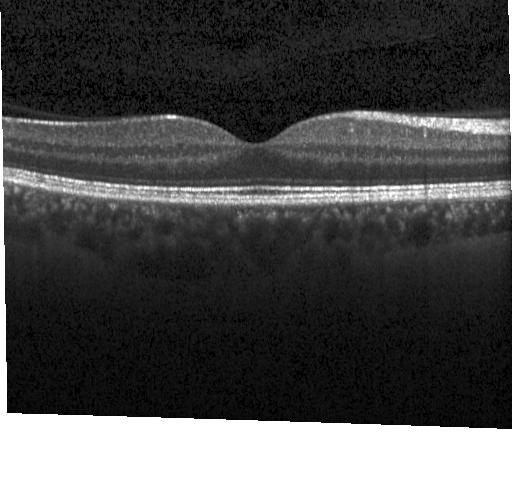

Macular OCT: no CNV, DME, or drusen.